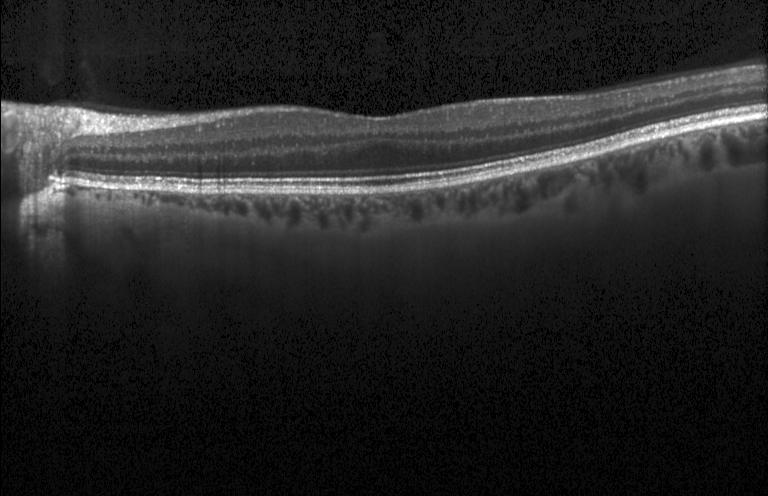

Acquired on a Heidelberg Spectralis, OCT line scan. This B-scan demonstrates neither CNV, DME, nor drusen.